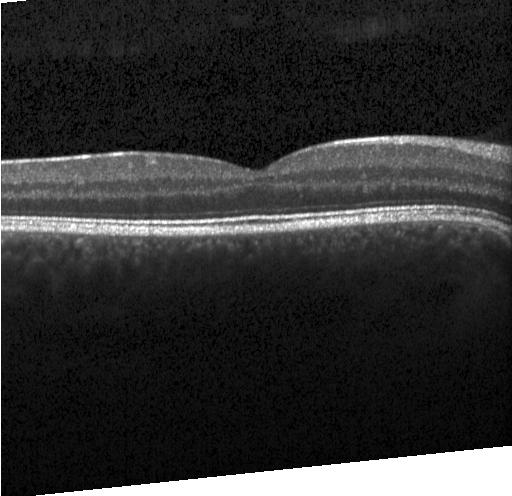

OCT line scan. Dx: no choroidal neovascularization, no diabetic macular edema, and no drusen.